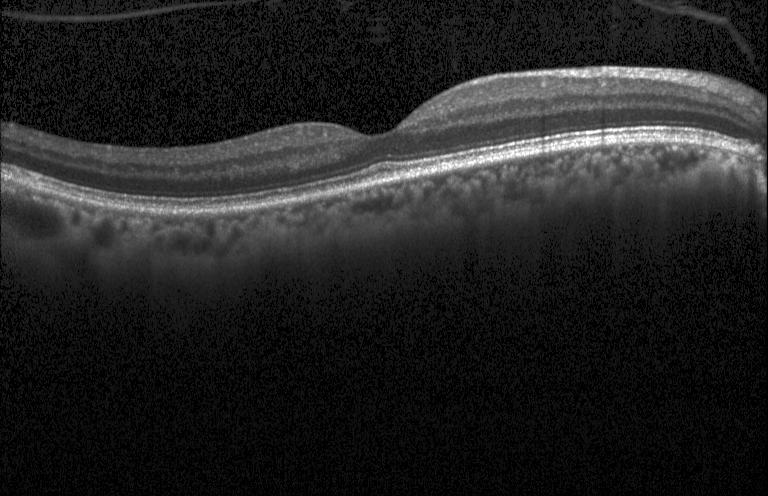
Retinal OCT cross-section; Heidelberg Spectralis. Diagnosis: no choroidal neovascularization, no diabetic macular edema, and no drusen.